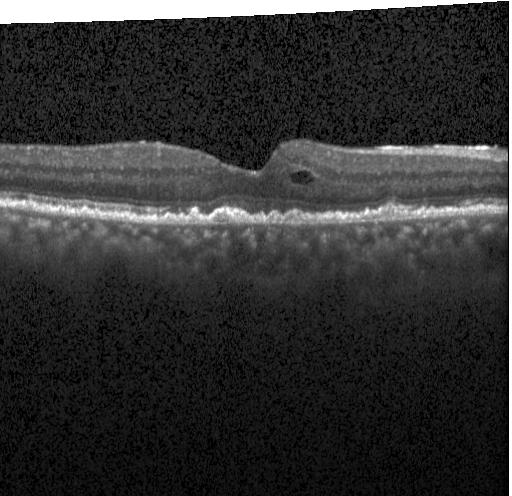

Macular scan, spectral-domain OCT, Heidelberg Spectralis OCT system, OCT B-scan — Macular OCT: a choroidal neovascular membrane.